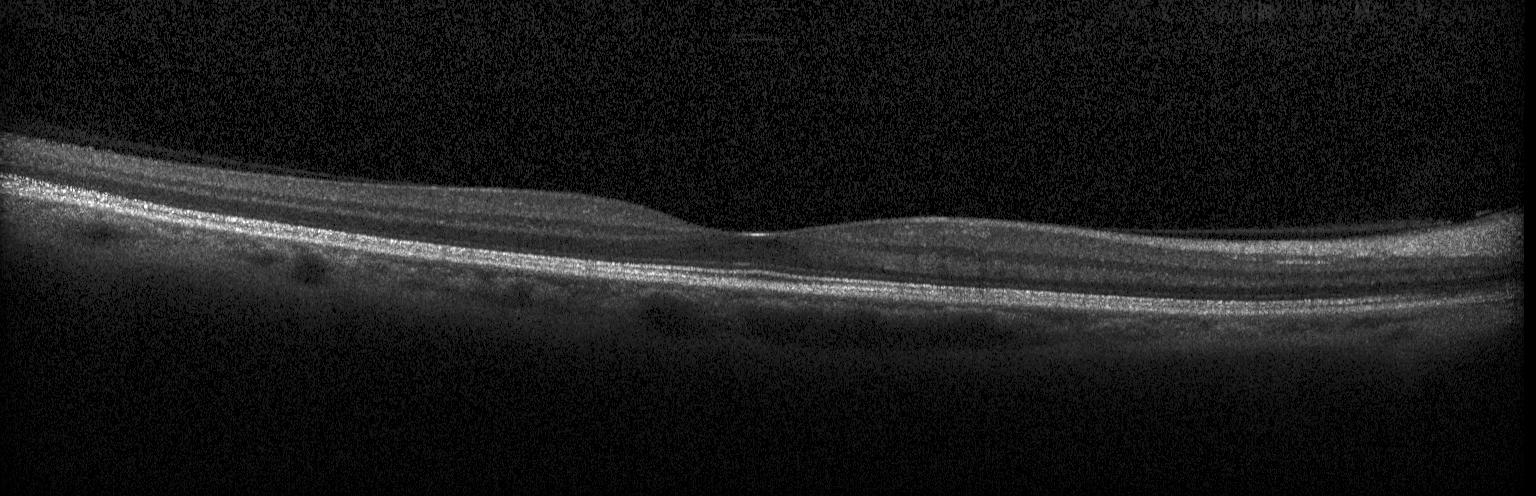 Retinal OCT B-scan
Dx: neither choroidal neovascularization, diabetic macular edema, nor drusen.